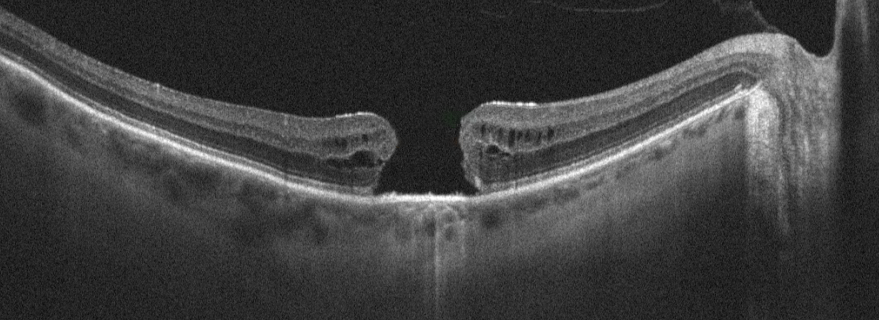

This B-scan demonstrates vitreomacular interface disease.